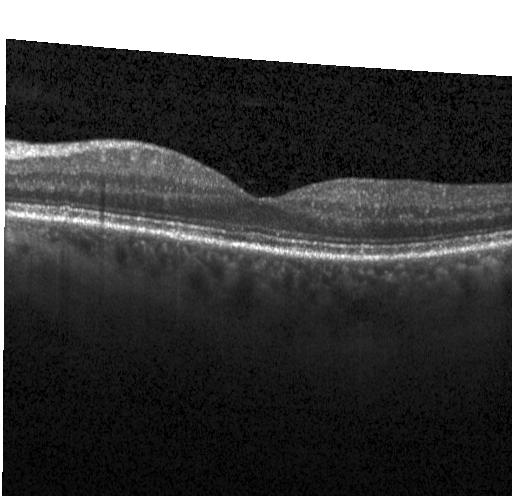 OCT B-scan — Finding: no CNV, no DME, and no drusen.